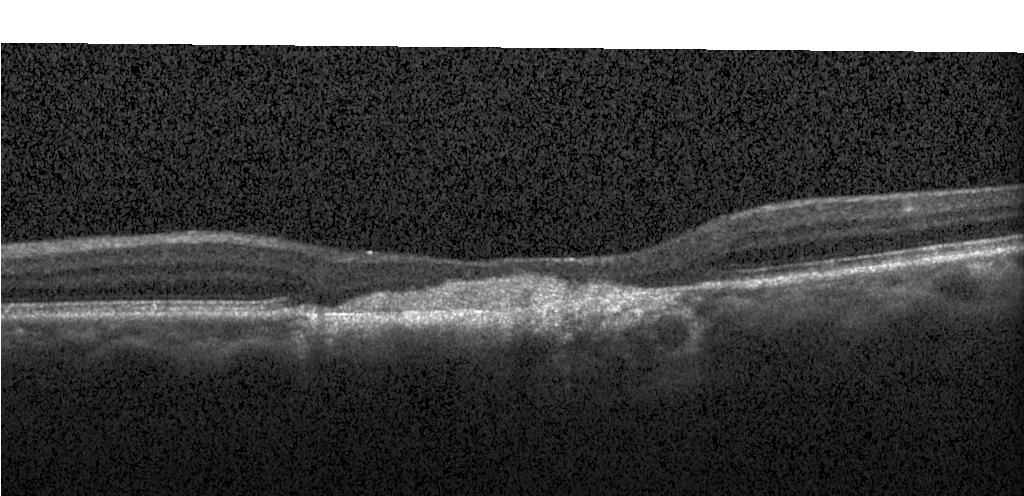
Retinal OCT B-scan. Finding: choroidal neovascularization.